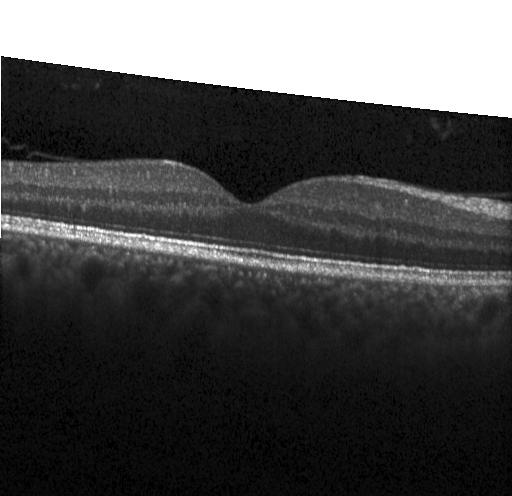
Optical coherence tomography B-scan. Spectral-domain OCT. Centered on the fovea. OCT finding: neither choroidal neovascularization, diabetic macular edema, nor drusen.